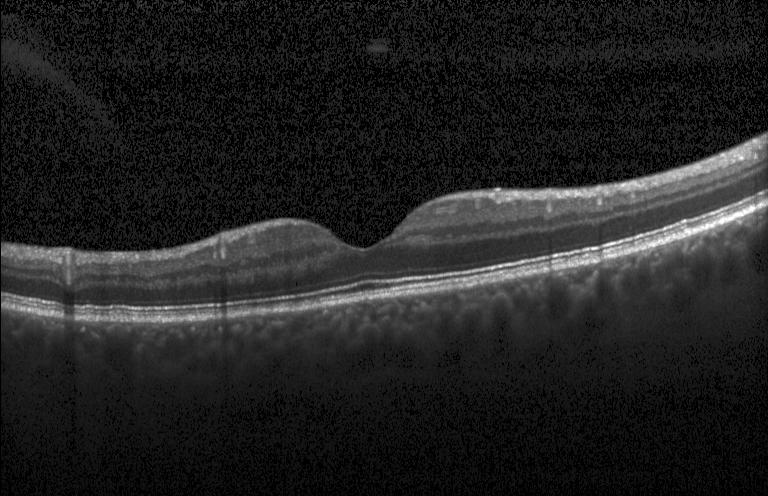
Impression: neither CNV, DME, nor drusen.